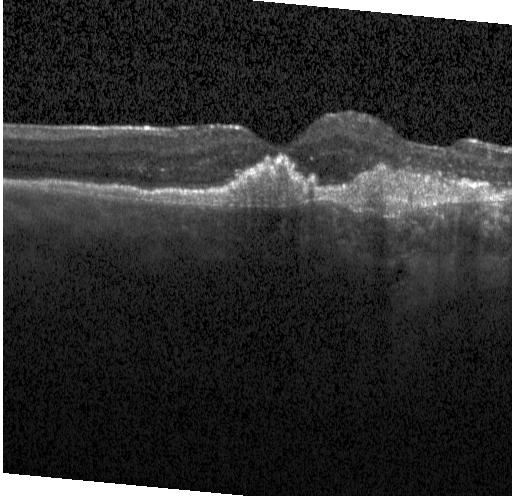
The scan shows CNV.